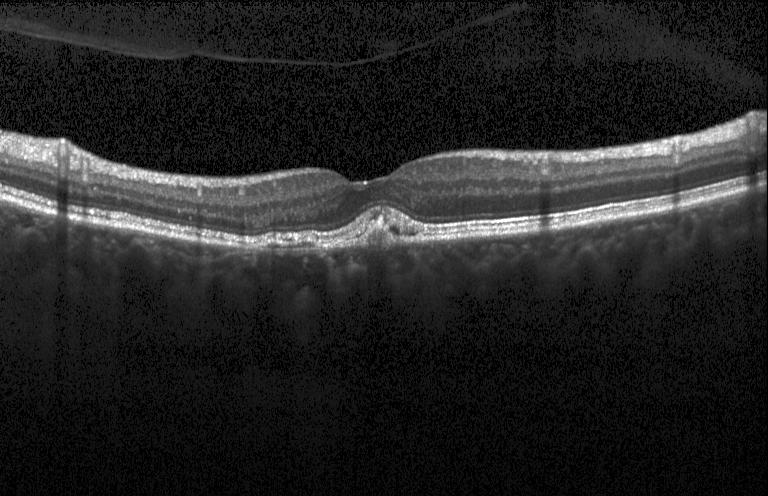
Finding: drusen.